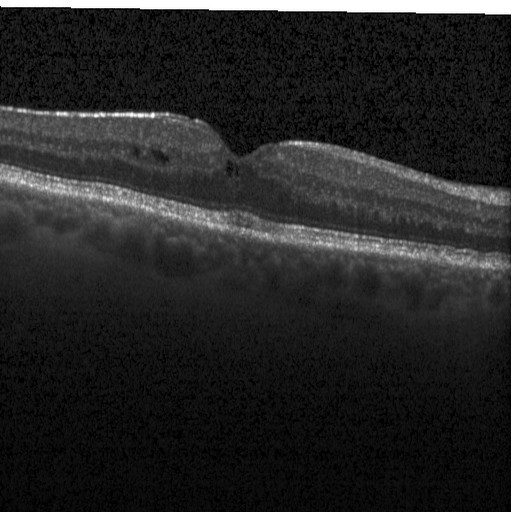 Through the macula; instrument: Heidelberg Spectralis; SD-OCT; OCT line scan. Diabetic macular edema (DME).